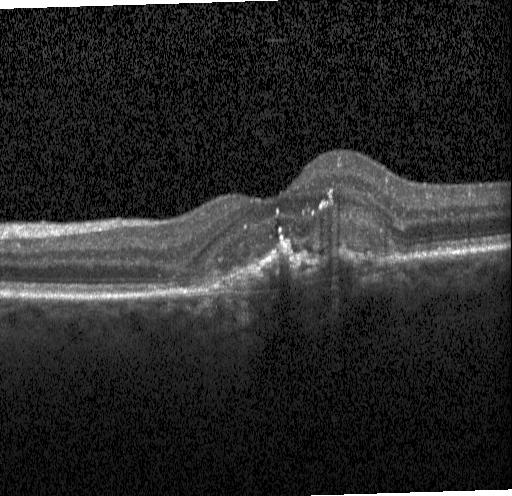

Optical coherence tomography B-scan. Spectral-domain optical coherence tomography.
The scan shows choroidal neovascularization.